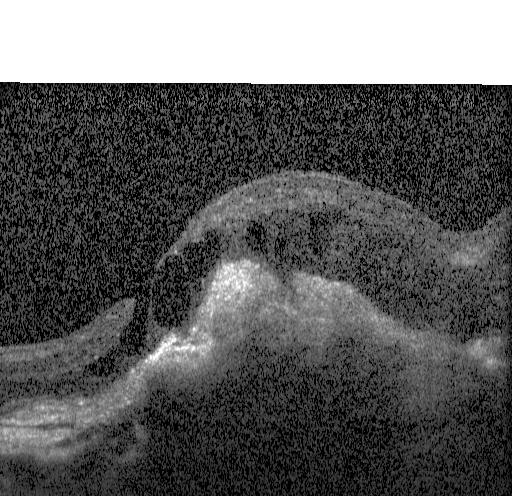 A choroidal neovascular membrane.